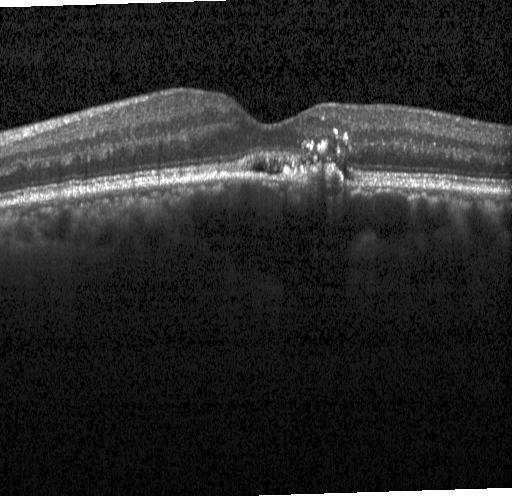

Finding: a choroidal neovascular membrane.